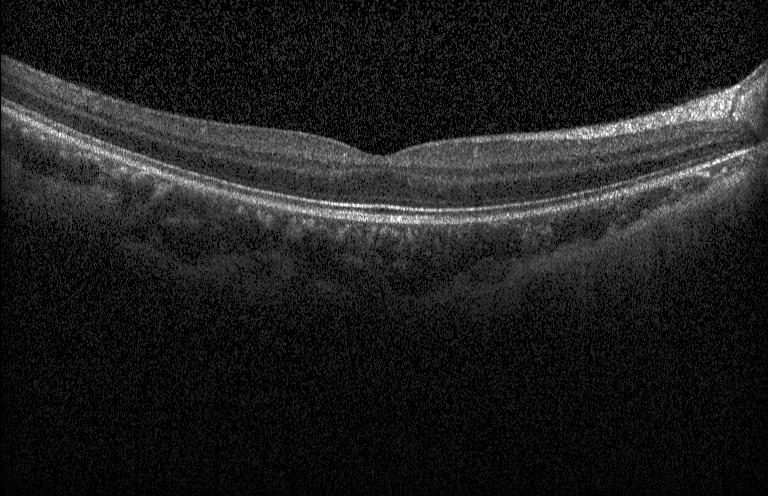

Dx: no choroidal neovascularization, no diabetic macular edema, and no drusen.